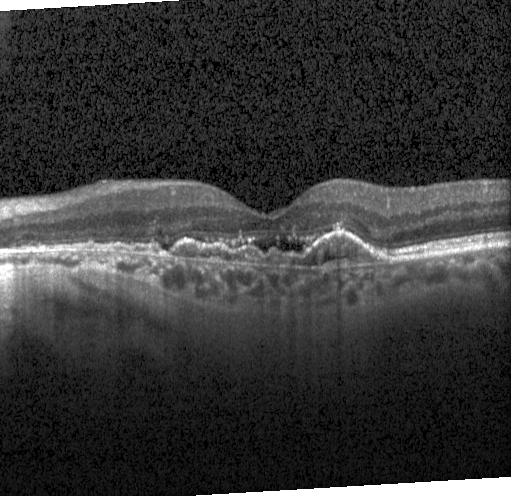
Centered on the fovea · retinal OCT cross-section · spectral-domain optical coherence tomography.
Diagnosis: CNV.